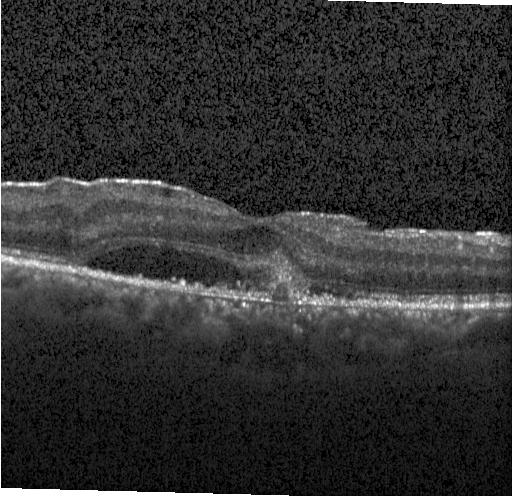

Optical coherence tomography scan. Heidelberg Spectralis OCT system. Spectral-domain optical coherence tomography. Diagnosis: a choroidal neovascular membrane.